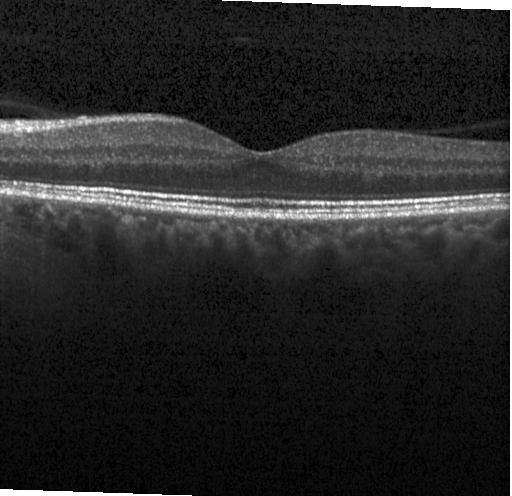

Acquired on a Heidelberg Spectralis · optical coherence tomography scan · spectral-domain OCT — The scan shows no CNV, no DME, and no drusen.